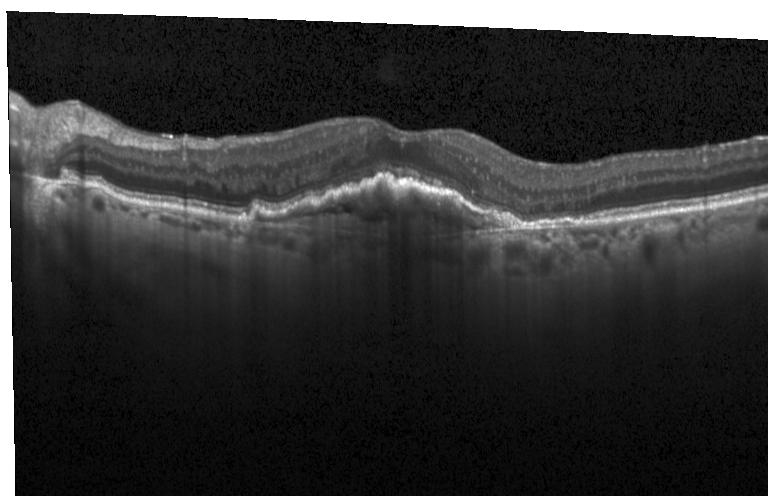
OCT scan showing a choroidal neovascular membrane.